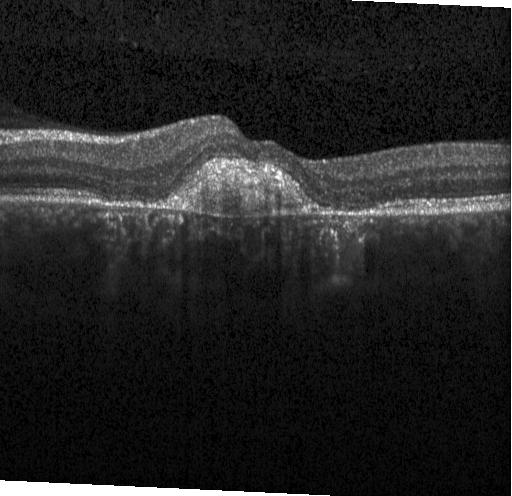
SD-OCT. Heidelberg Spectralis OCT system. Retinal OCT B-scan. Horizontal scan through the fovea — Dx: a choroidal neovascular membrane.